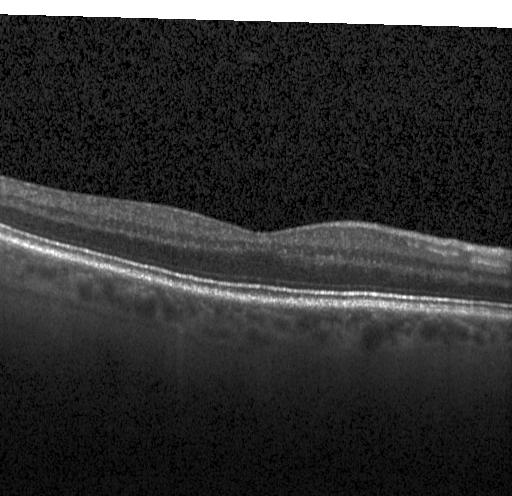

Finding: neither choroidal neovascularization, diabetic macular edema, nor drusen.